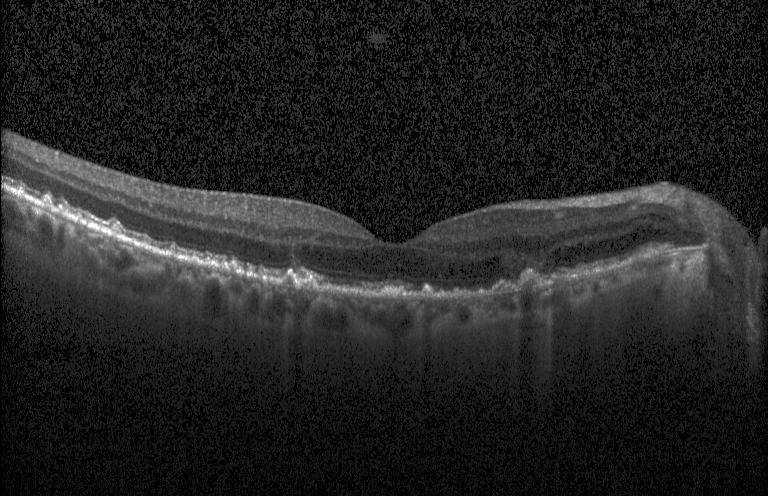 Impression: multiple drusen.